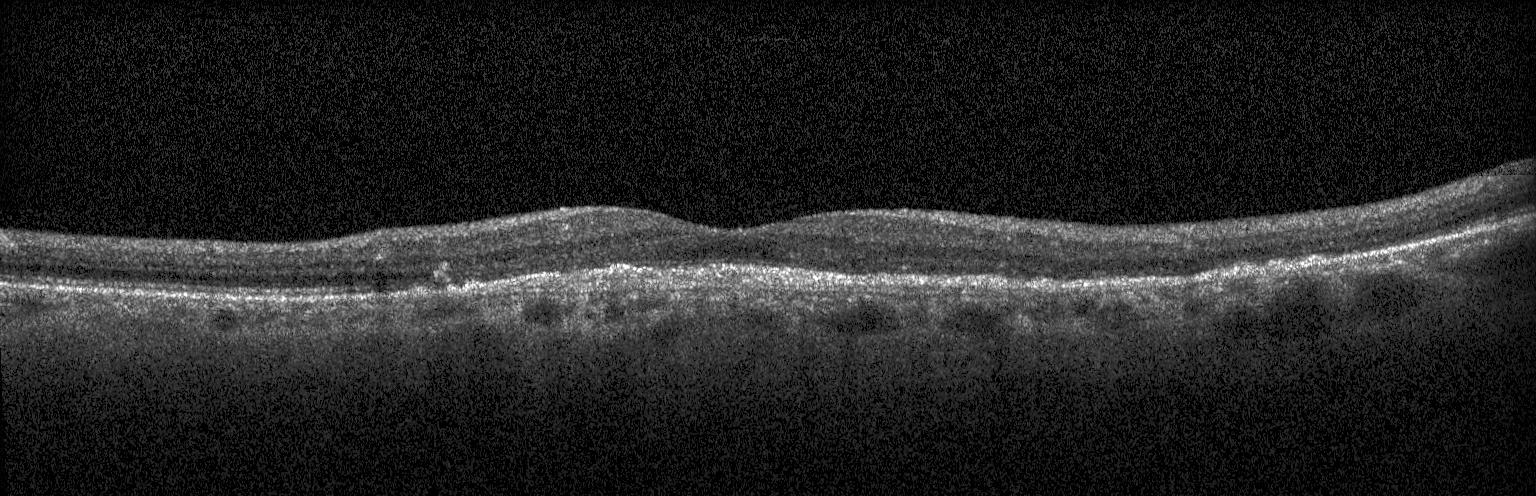
Optical coherence tomography scan, acquired on a Heidelberg Spectralis, spectral-domain OCT — Finding: a choroidal neovascular membrane.